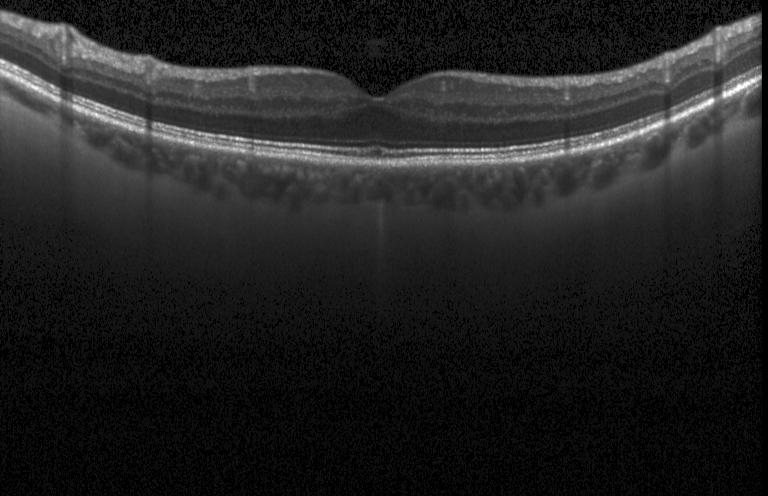

OCT line scan — Assessment: neither choroidal neovascularization, diabetic macular edema, nor drusen.